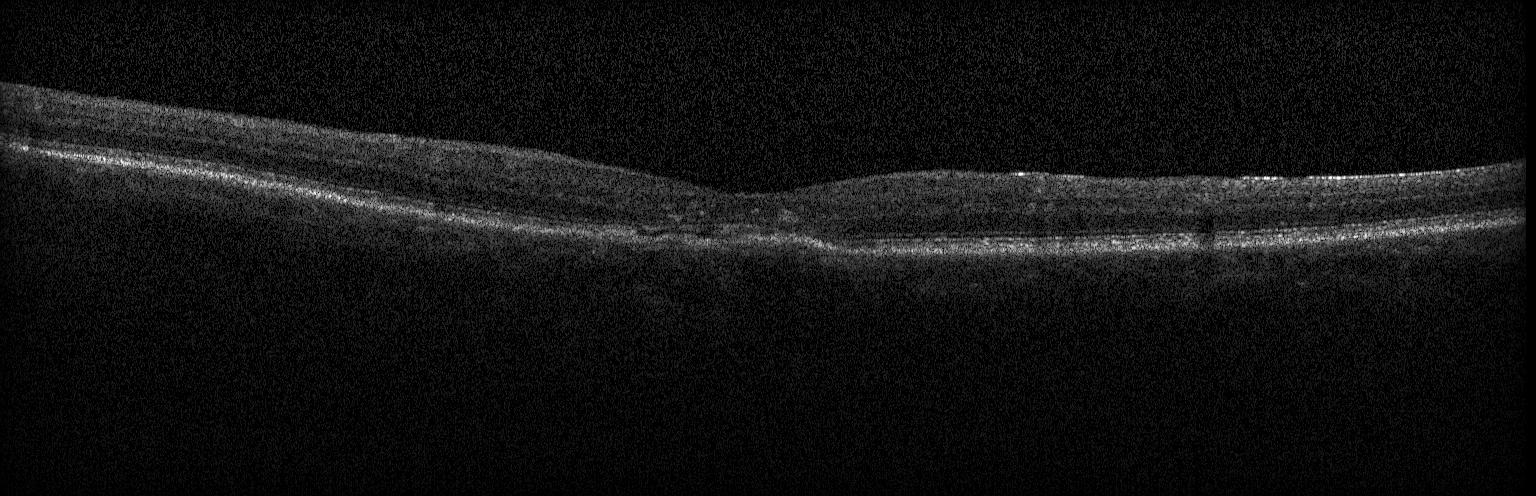

CNV.